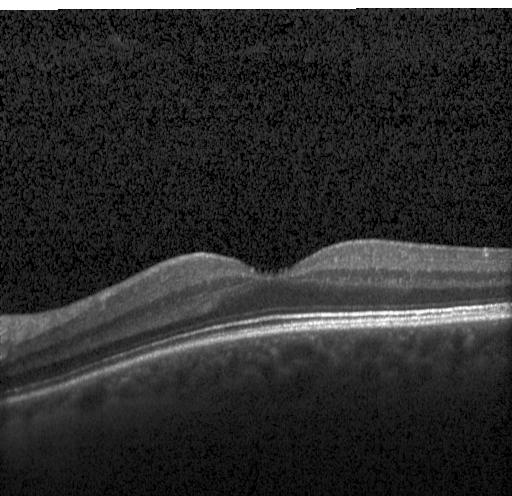

Retinal OCT cross-section — Assessment: no choroidal neovascularization, no diabetic macular edema, and no drusen.